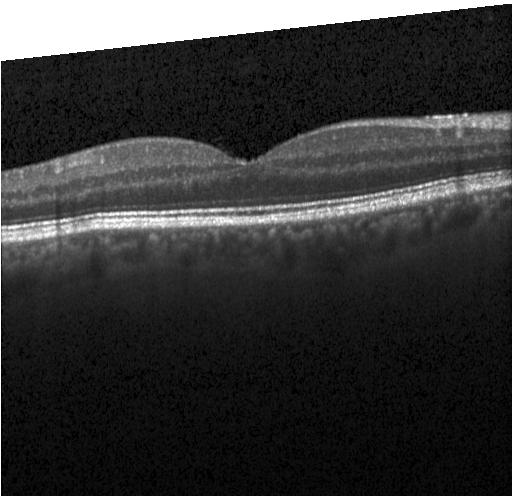
Spectral-domain optical coherence tomography · optical coherence tomography scan · horizontal scan through the fovea.
Finding: neither choroidal neovascularization, diabetic macular edema, nor drusen.